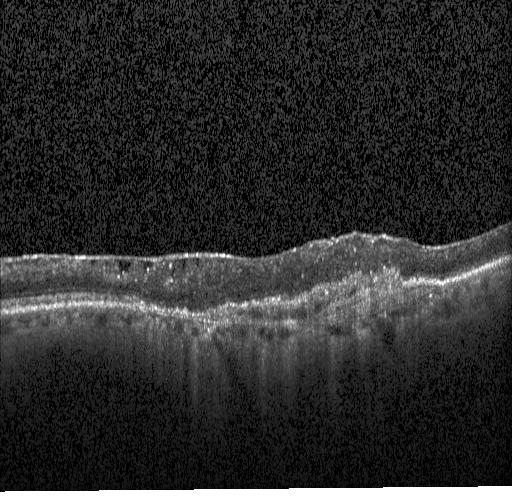 Retinal OCT cross-section
Finding: a choroidal neovascular membrane.